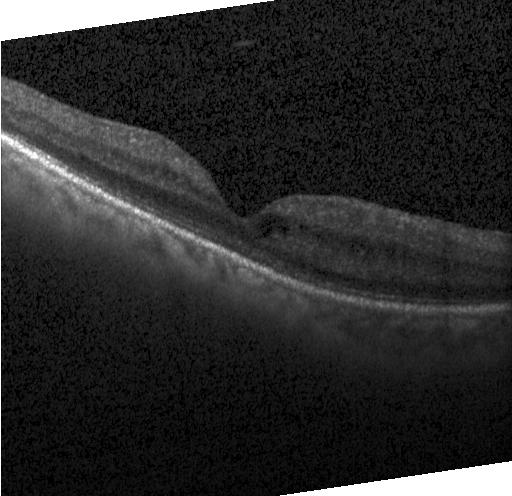 OCT scan showing DME.